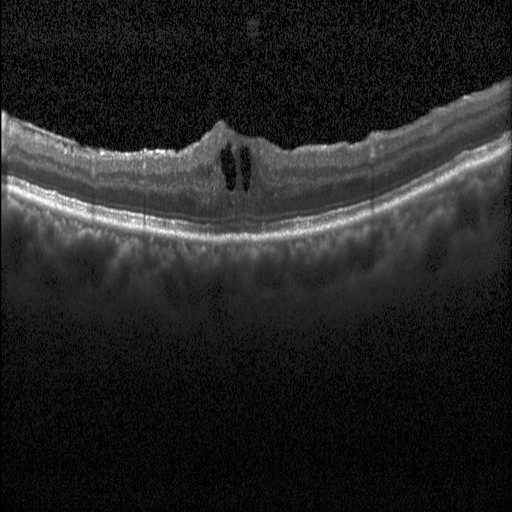
SD-OCT; retinal OCT B-scan — OCT finding: diabetic macular edema.